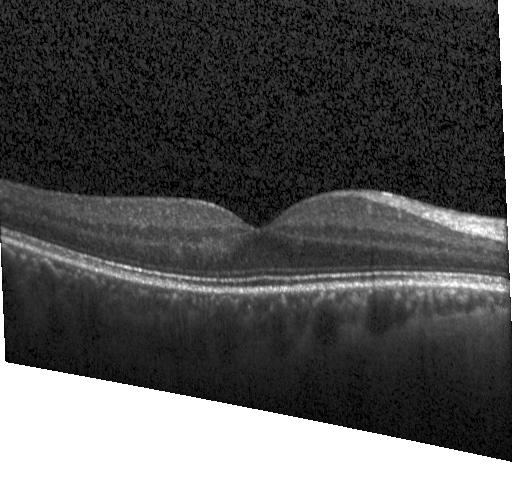

Retinal OCT B-scan · Heidelberg Spectralis OCT system. The scan shows no CNV, no DME, and no drusen.